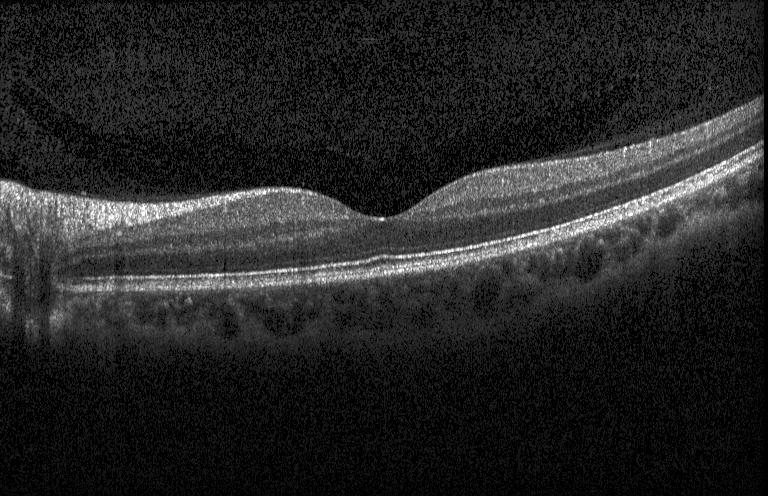 Diagnosis: no choroidal neovascularization, diabetic macular edema, or drusen.